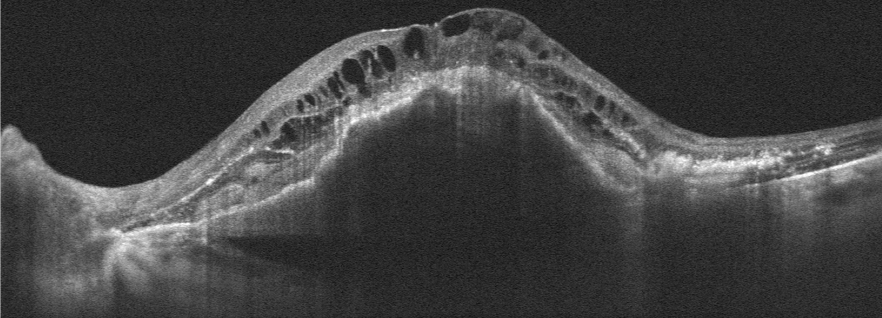

Finding: age-related macular degeneration (AMD).